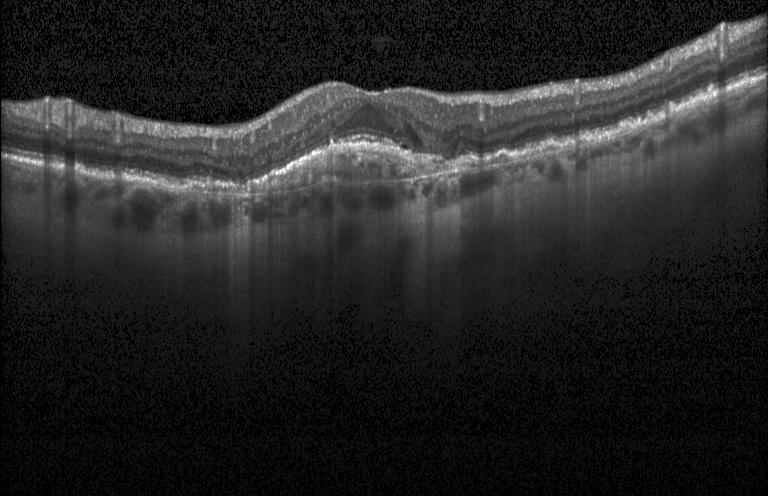 Retinal OCT cross-section. Acquired on a Heidelberg Spectralis. Horizontal scan through the fovea — This B-scan demonstrates choroidal neovascularization (CNV).